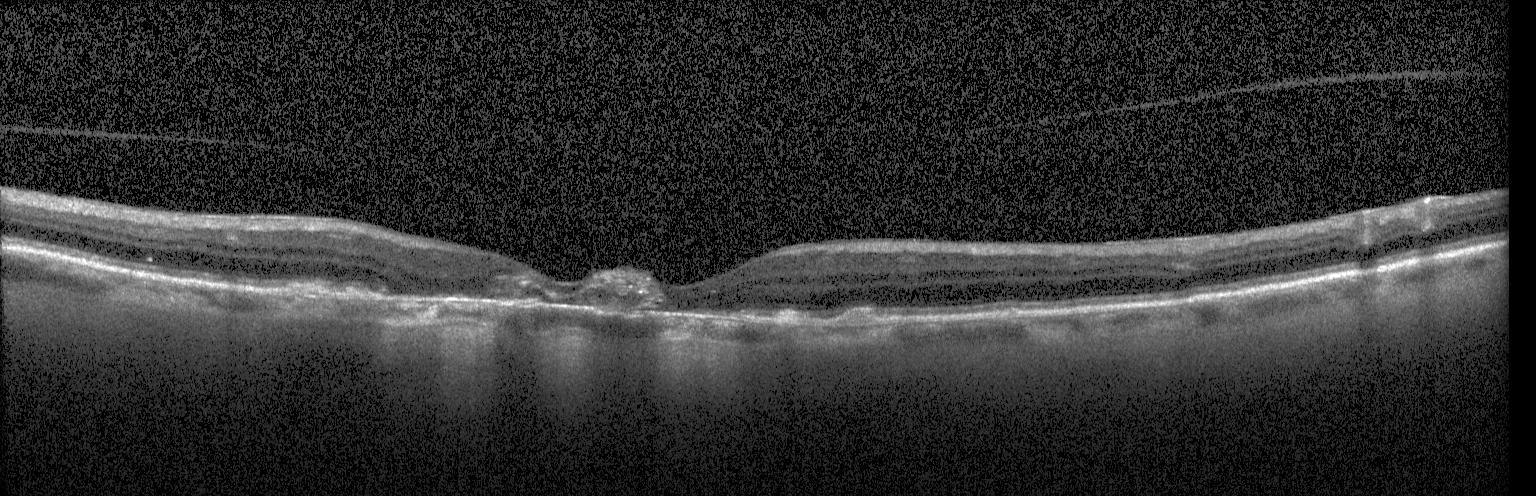

Macular OCT: a choroidal neovascular membrane.